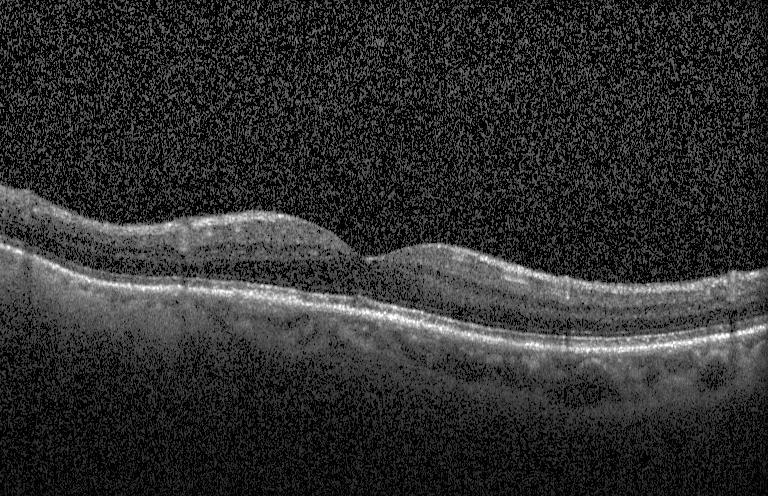 Optical coherence tomography scan · macular scan · spectral-domain OCT · instrument: Heidelberg Spectralis — Impression: no CNV, no DME, and no drusen.